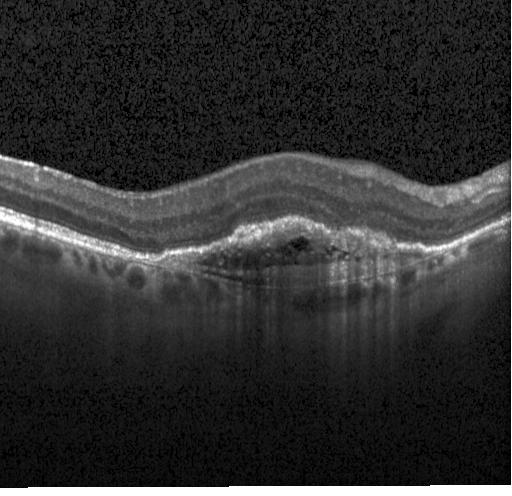

OCT finding: choroidal neovascularization.